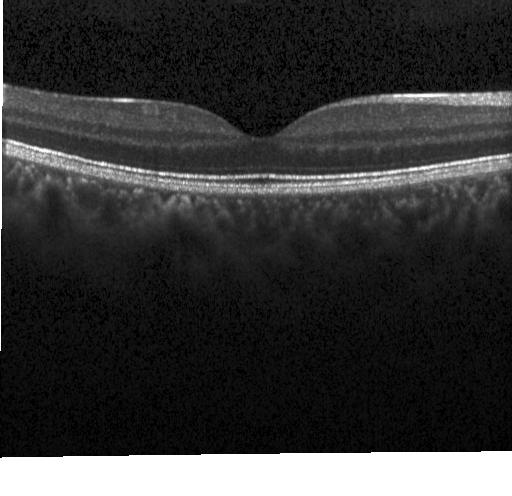

Fovea-centered; SD-OCT; acquired on a Heidelberg Spectralis; retinal OCT cross-section — OCT finding: no evidence of CNV, DME, or drusen.